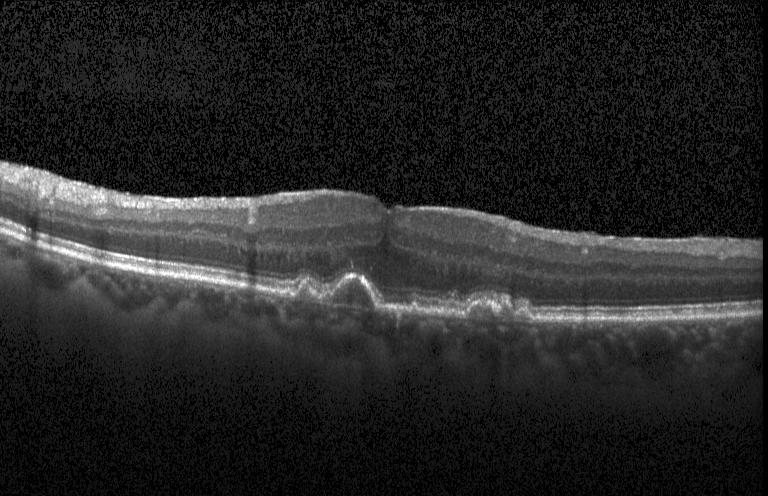

SD-OCT · through the macula · retinal OCT cross-section · Heidelberg Spectralis OCT system — Macular OCT: a choroidal neovascular membrane.